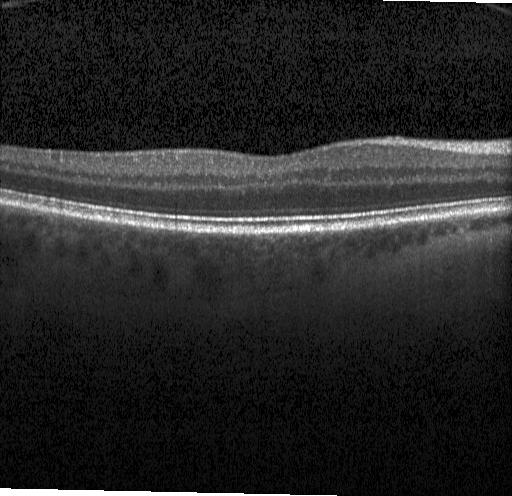 Macular scan. Spectral-domain OCT. OCT line scan. The scan shows neither choroidal neovascularization, diabetic macular edema, nor drusen.